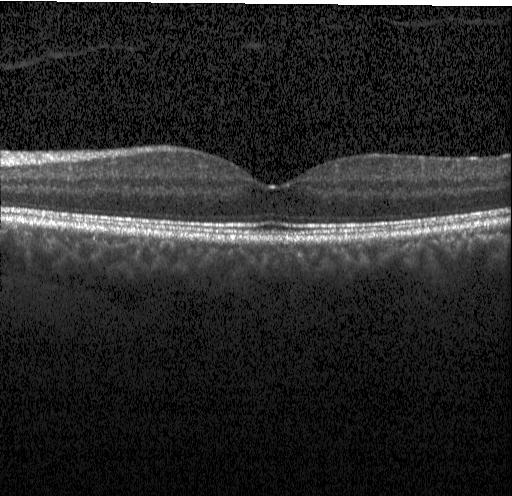 OCT B-scan, macular scan.
The scan shows neither choroidal neovascularization, diabetic macular edema, nor drusen.